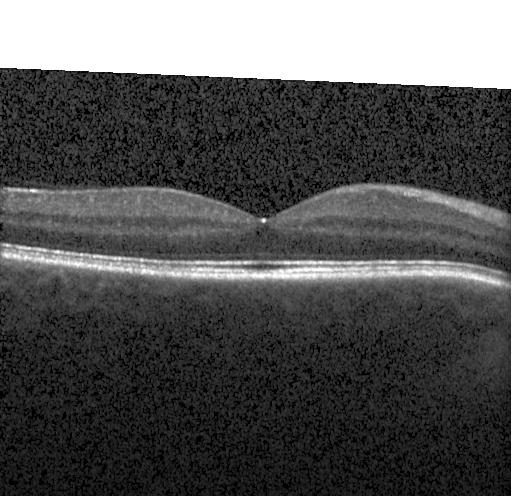 Spectral-domain optical coherence tomography, instrument: Heidelberg Spectralis, OCT B-scan, fovea-centered — Assessment: no choroidal neovascularization, no diabetic macular edema, and no drusen.